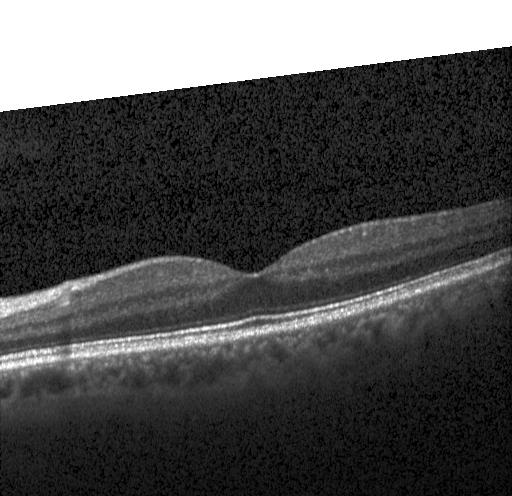
OCT B-scan, spectral-domain OCT. OCT finding: neither CNV, DME, nor drusen.